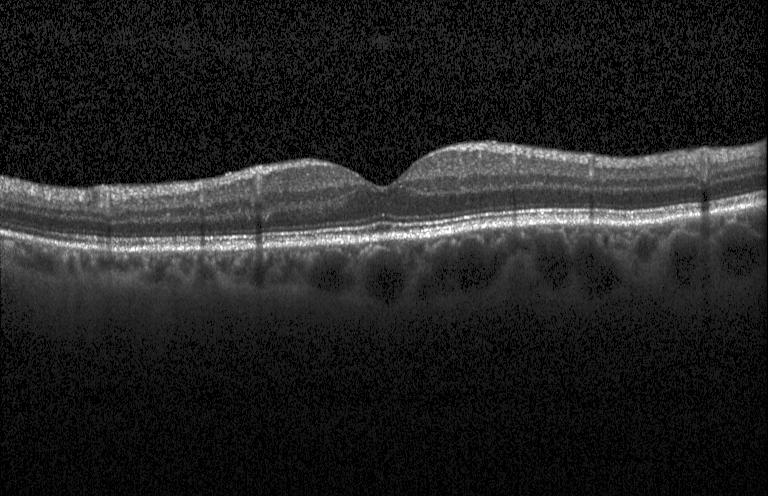
Optical coherence tomography B-scan; spectral-domain optical coherence tomography — Finding: neither choroidal neovascularization, diabetic macular edema, nor drusen.